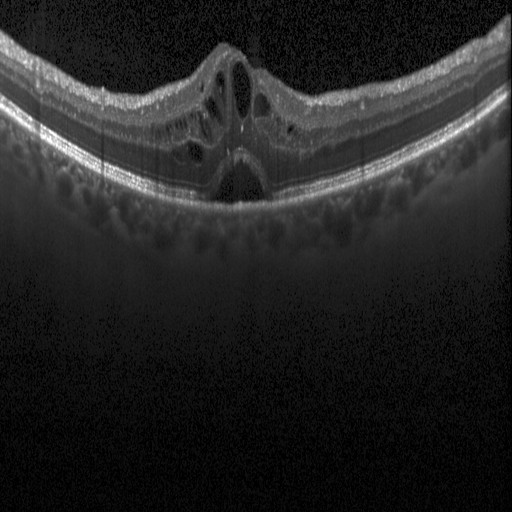
Optical coherence tomography scan; instrument: Heidelberg Spectralis; macular scan; spectral-domain optical coherence tomography.
Finding: diabetic macular edema.